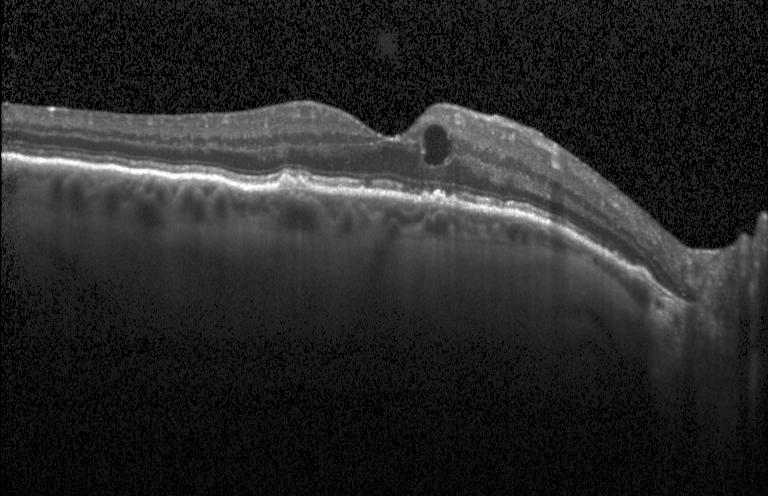

Impression: choroidal neovascularization (CNV).